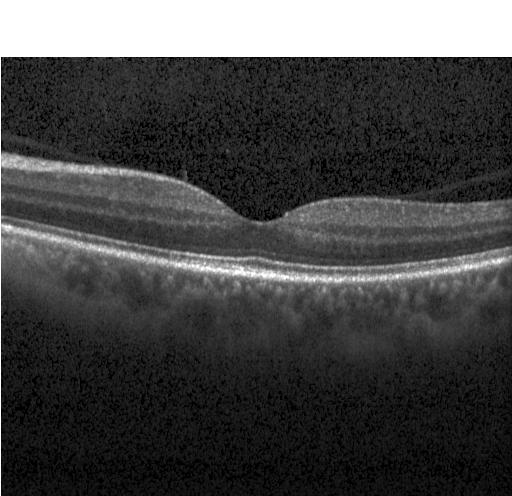
Horizontal scan through the fovea. Spectral-domain optical coherence tomography. OCT line scan. Heidelberg Spectralis
Diagnosis: no choroidal neovascularization, no diabetic macular edema, and no drusen.